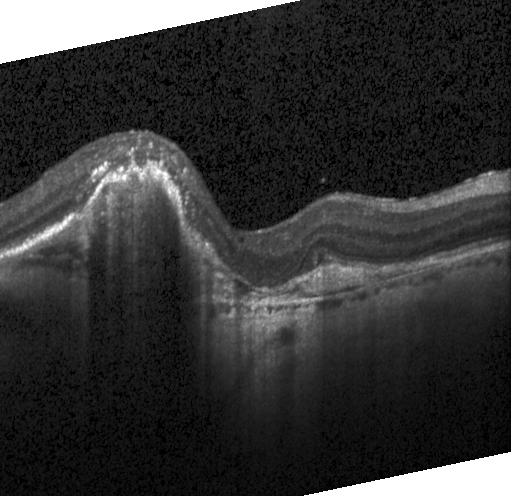

Retinal OCT cross-section
The scan shows a choroidal neovascular membrane.